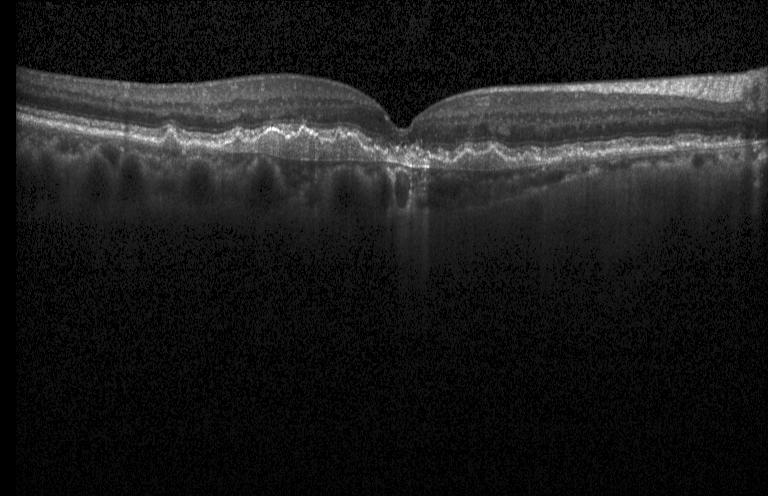

Optical coherence tomography scan
Diagnosis: choroidal neovascularization.